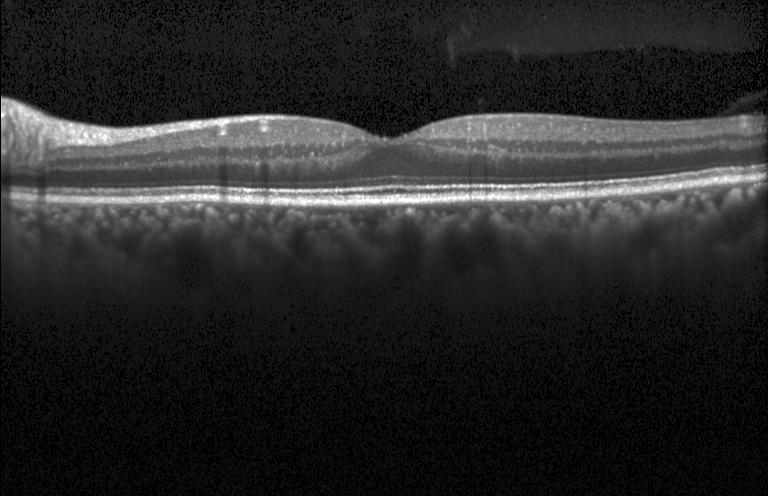 Impression: no evidence of choroidal neovascularization, diabetic macular edema, or drusen.